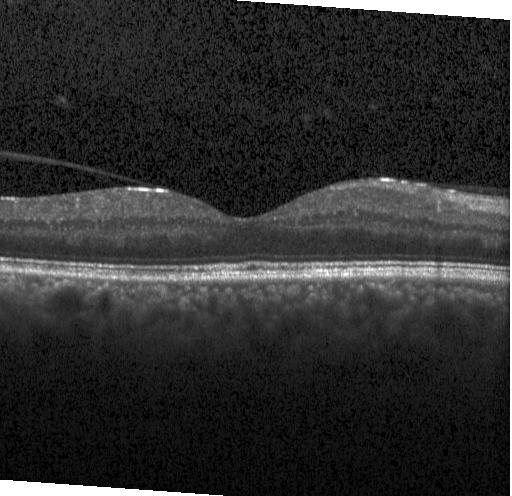
Optical coherence tomography B-scan, SD-OCT, horizontal scan through the fovea, instrument: Heidelberg Spectralis
This B-scan demonstrates no CNV, DME, or drusen.